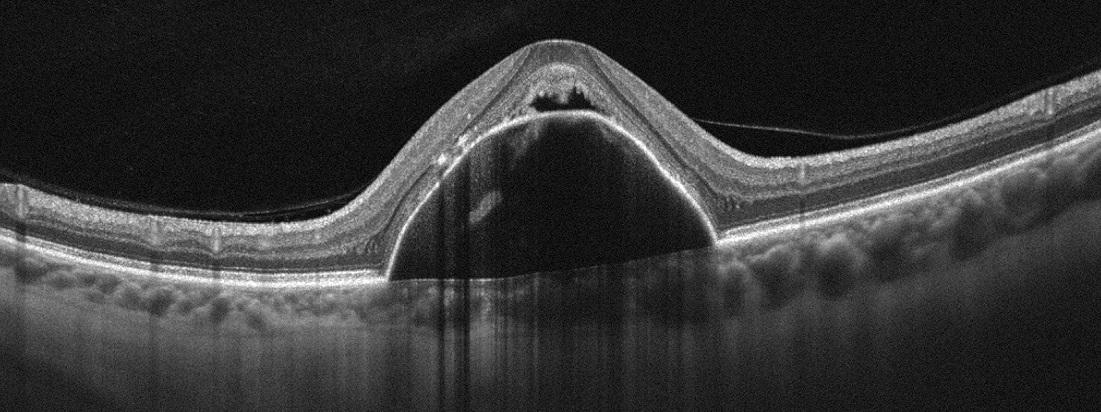 Optical coherence tomography scan. Finding: age-related macular degeneration (AMD).